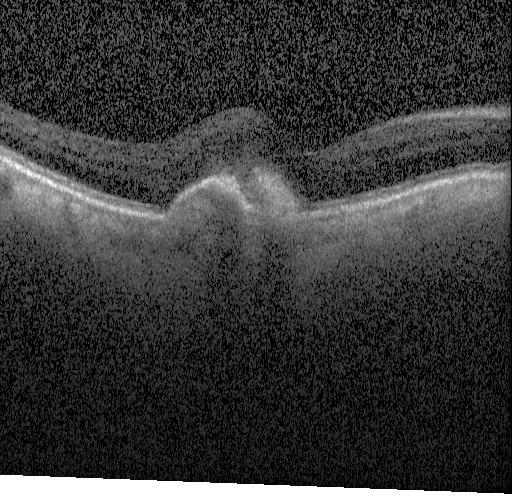
OCT finding: choroidal neovascularization (CNV).